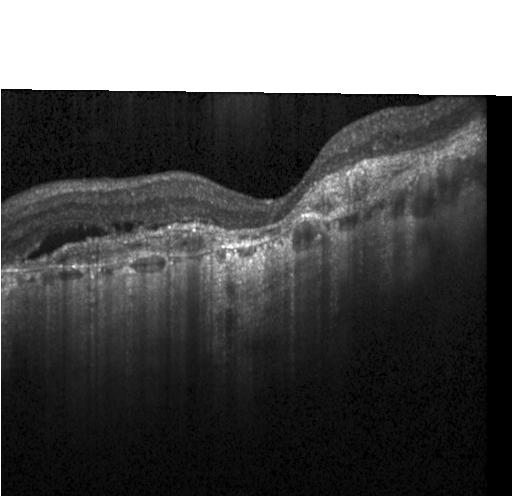

Assessment: choroidal neovascularization (CNV).